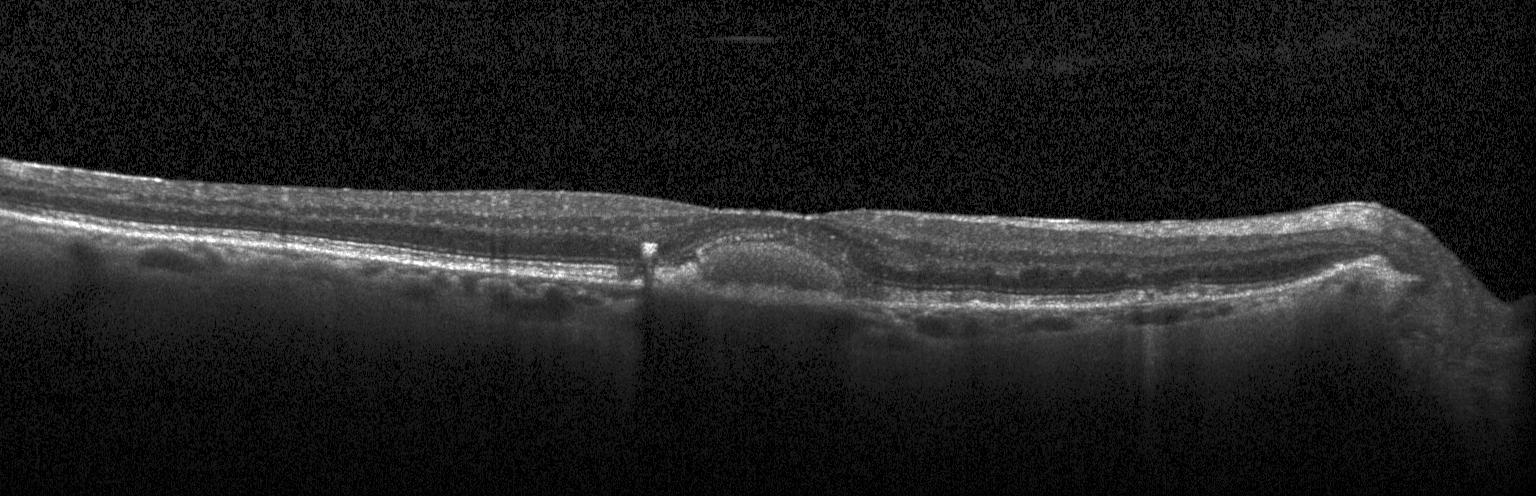
Heidelberg Spectralis, retinal OCT B-scan.
Finding: choroidal neovascularization (CNV).